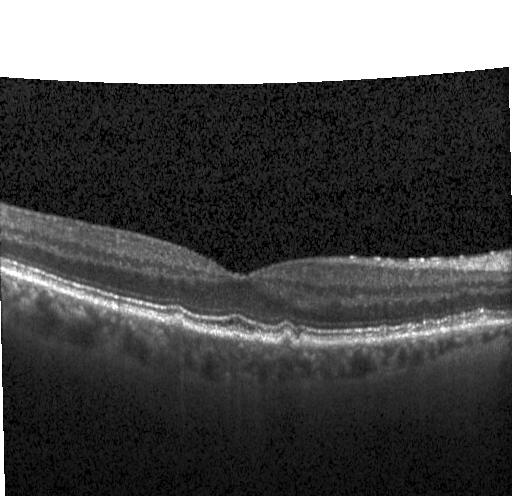
Diagnosis: multiple drusen.